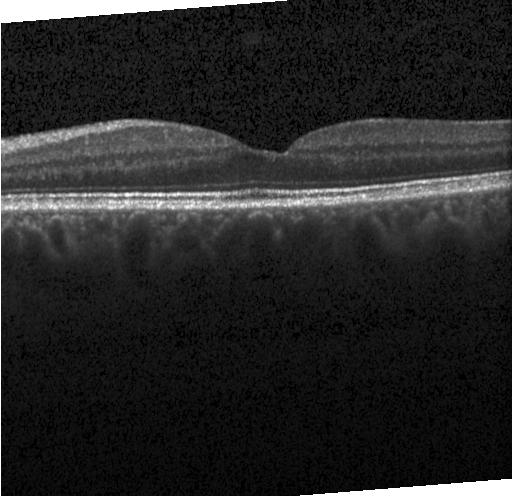
The scan shows no evidence of choroidal neovascularization, diabetic macular edema, or drusen.